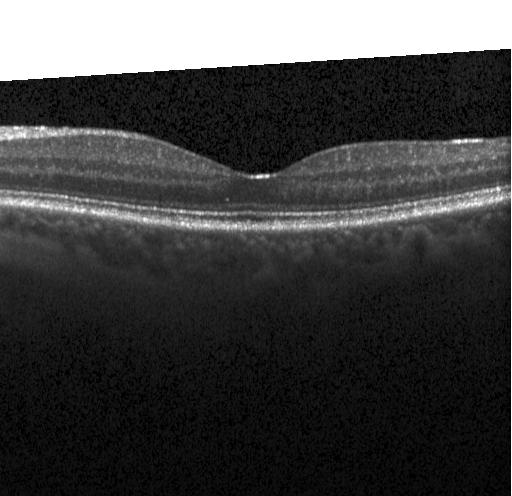

OCT scan showing no evidence of choroidal neovascularization, diabetic macular edema, or drusen.